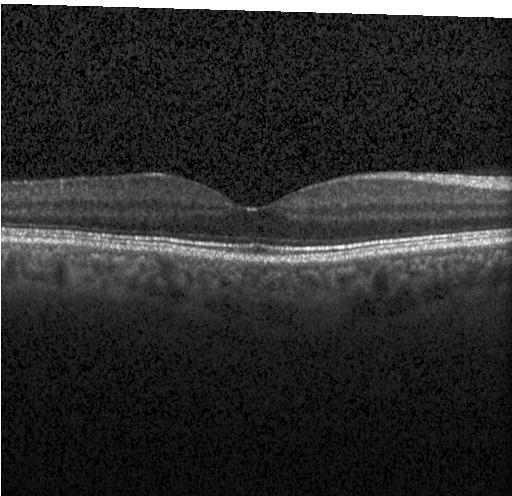 Diagnosis: no choroidal neovascularization, diabetic macular edema, or drusen.